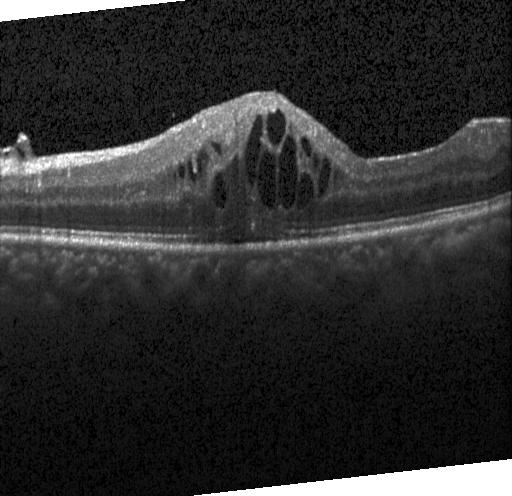

Optical coherence tomography scan. OCT finding: diabetic macular edema.